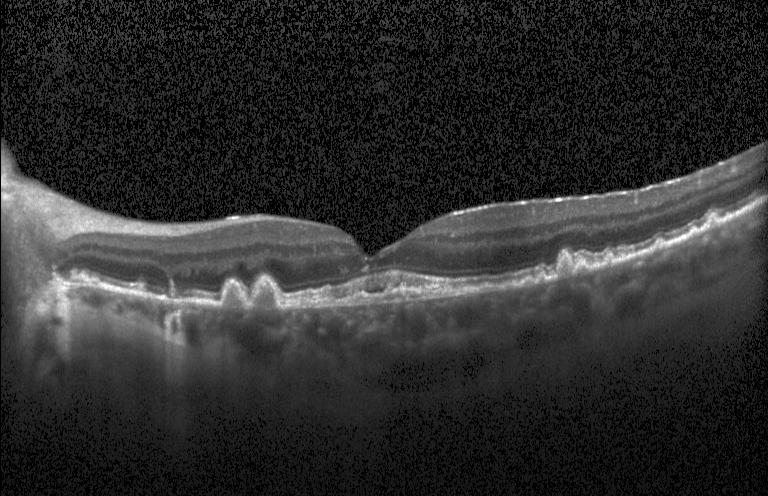
Optical coherence tomography B-scan — The scan shows choroidal neovascularization (CNV).